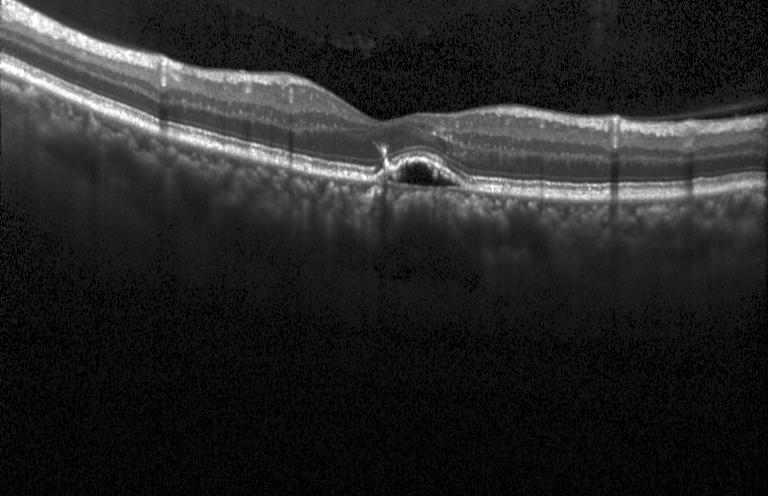 SD-OCT, horizontal scan through the fovea, OCT line scan.
Impression: a choroidal neovascular membrane.